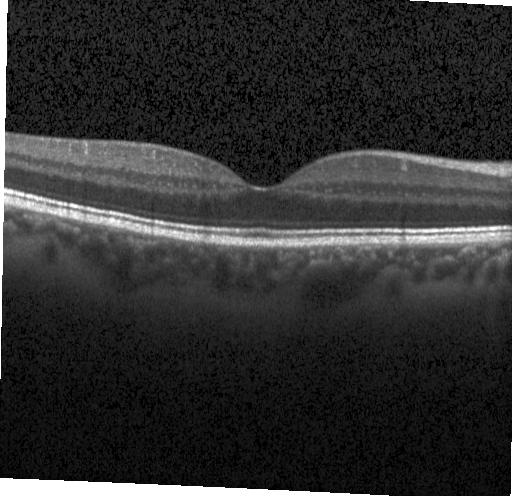

Retinal OCT B-scan
OCT finding: no choroidal neovascularization, no diabetic macular edema, and no drusen.